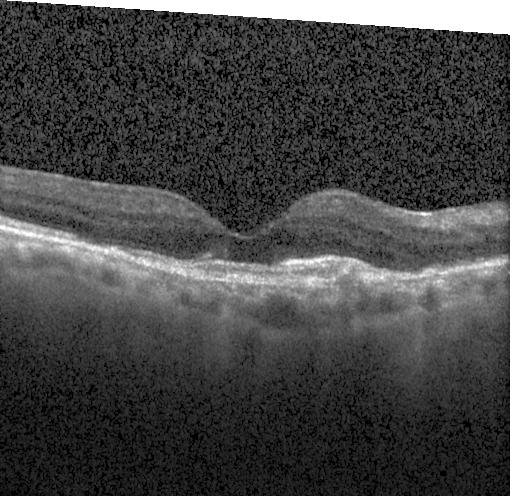

Heidelberg Spectralis; centered on the fovea; retinal OCT B-scan. The scan shows choroidal neovascularization.